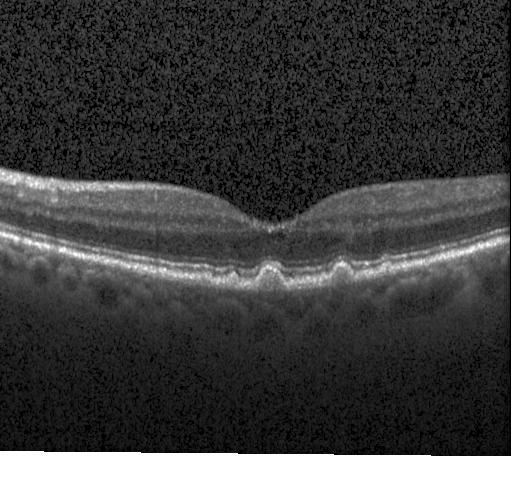

Optical coherence tomography scan — The scan shows sub-RPE drusenoid deposits.